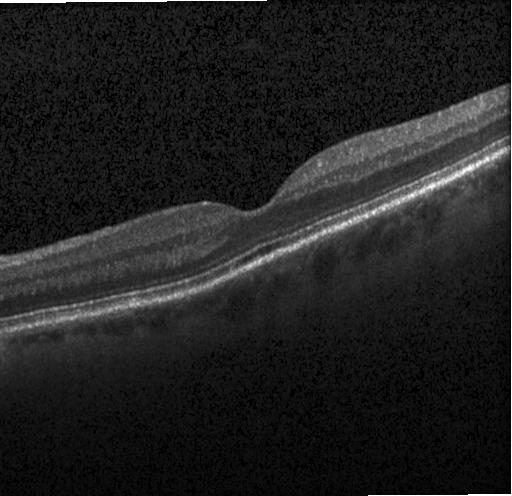
This B-scan demonstrates neither CNV, DME, nor drusen.